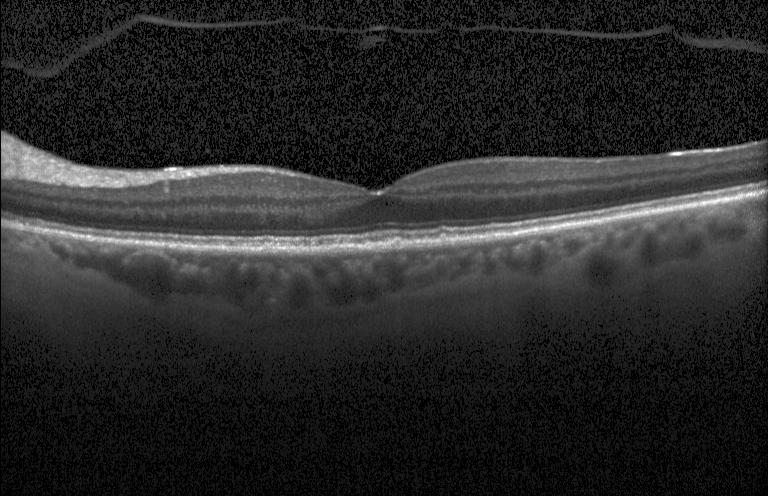 OCT finding: multiple drusen.